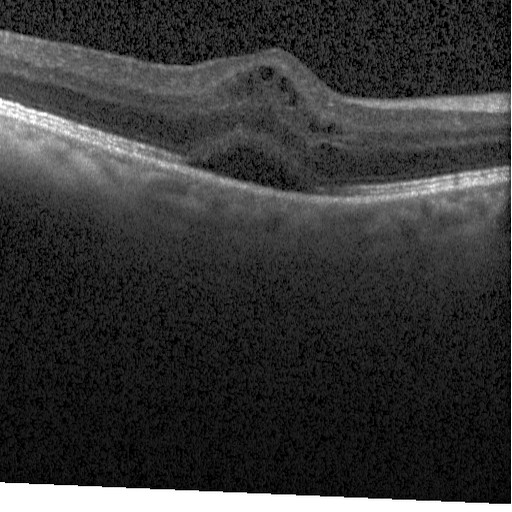 Diagnosis: DME.